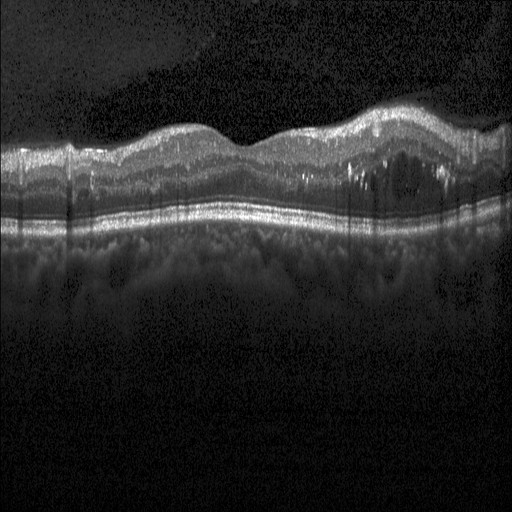

Diagnosis: diabetic macular edema (DME).